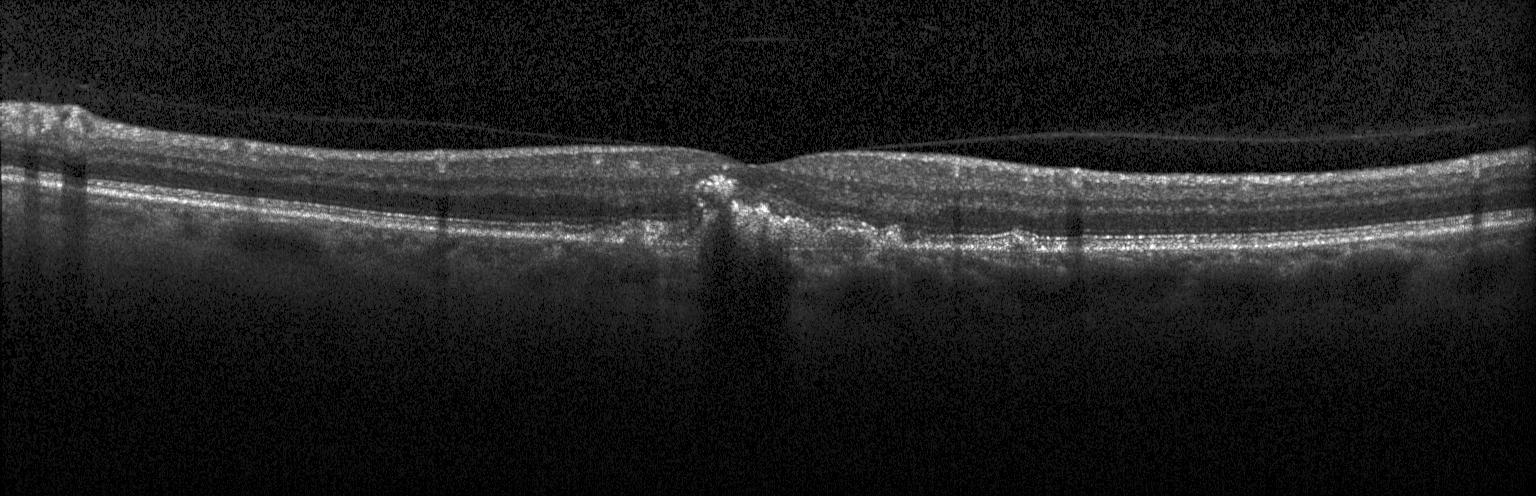 Spectral-domain optical coherence tomography. Retinal OCT B-scan. Impression: a choroidal neovascular membrane.